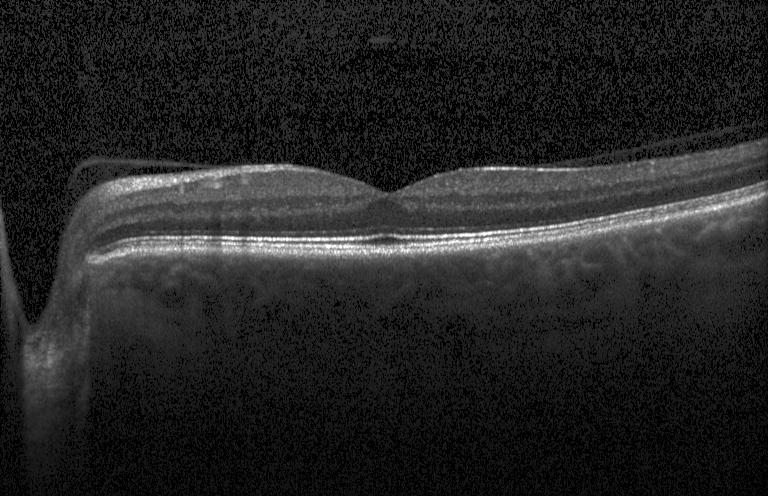 Spectral-domain optical coherence tomography · retinal OCT cross-section · Heidelberg Spectralis · horizontal scan through the fovea
OCT finding: neither CNV, DME, nor drusen.